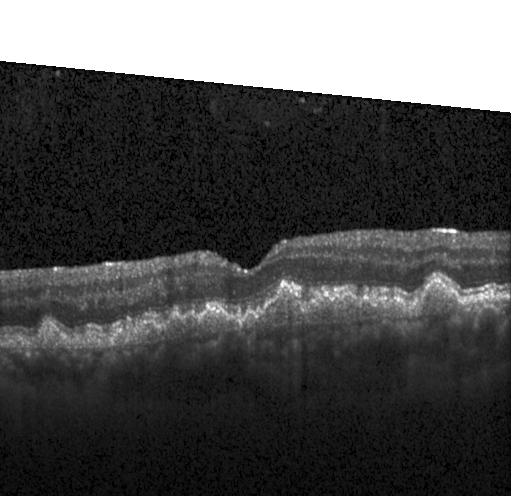 Retinal OCT cross-section — This B-scan demonstrates choroidal neovascularization.